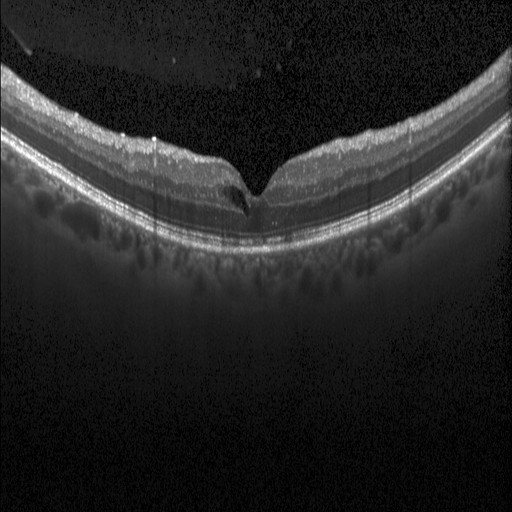 OCT B-scan, spectral-domain OCT, Heidelberg Spectralis OCT system, fovea-centered.
Finding: diabetic macular edema (DME).